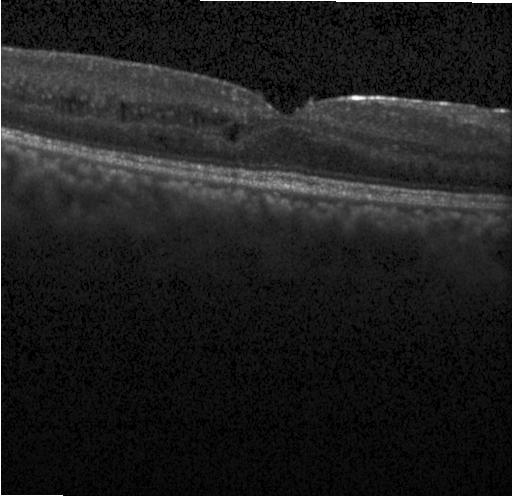
The scan shows DME.